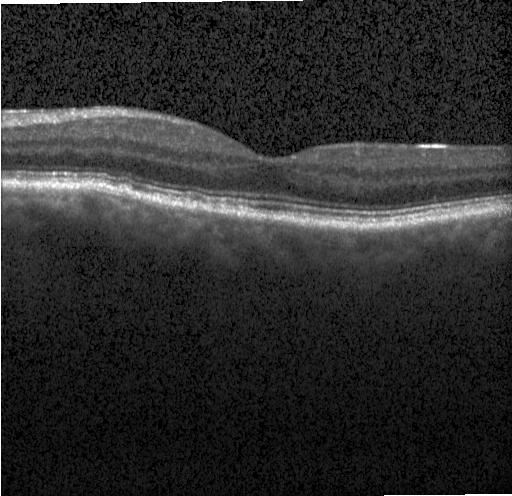
Retinal OCT cross-section — Impression: sub-RPE drusenoid deposits.